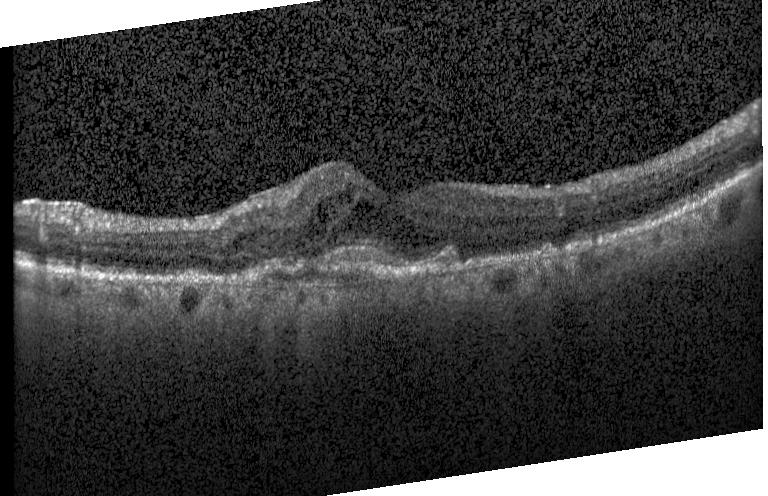

Through the macula; retinal OCT cross-section
Choroidal neovascularization.